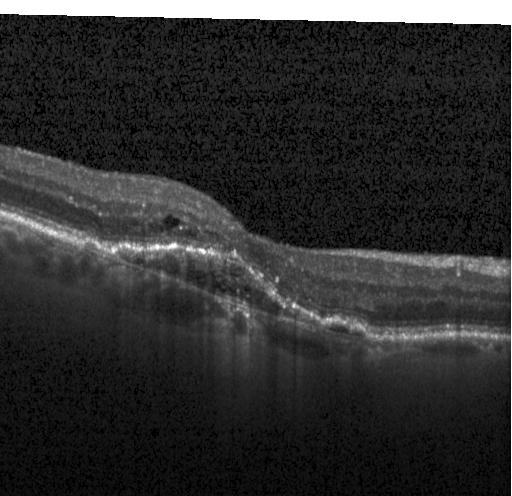

Diagnosis: choroidal neovascularization (CNV).